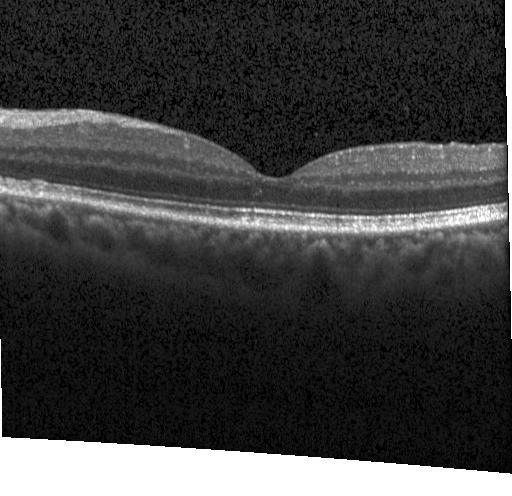
Optical coherence tomography B-scan · spectral-domain optical coherence tomography · fovea-centered — Neither choroidal neovascularization, diabetic macular edema, nor drusen.